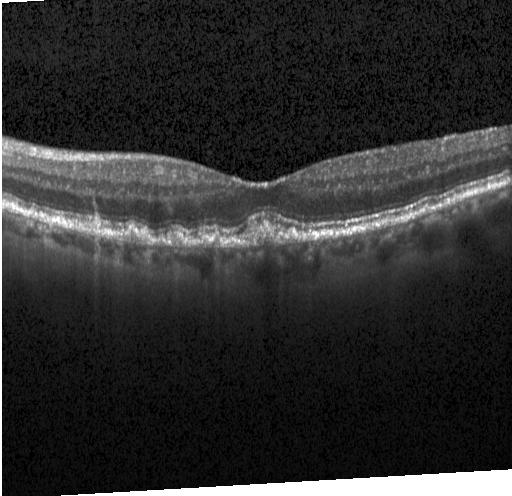 Assessment: sub-RPE drusenoid deposits.